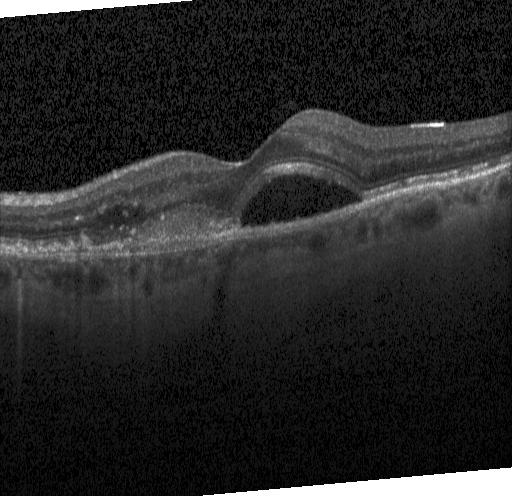
Retinal OCT B-scan, acquired on a Heidelberg Spectralis, SD-OCT, centered on the fovea — Finding: choroidal neovascularization.